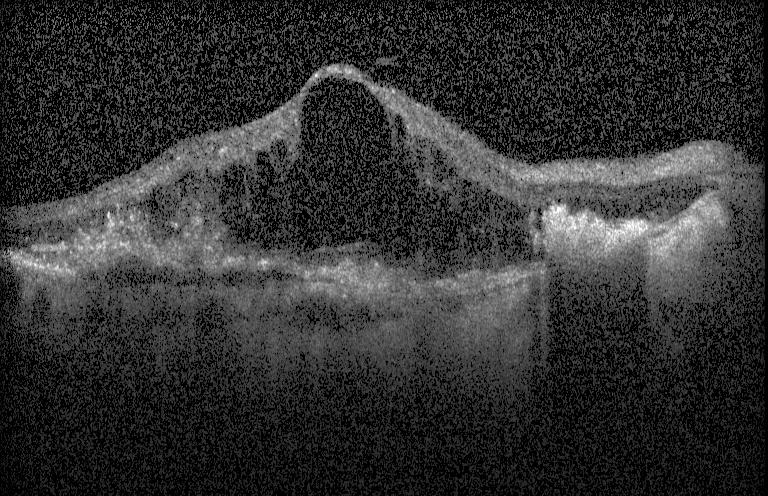
OCT B-scan; spectral-domain OCT; horizontal scan through the fovea
Impression: choroidal neovascularization (CNV).